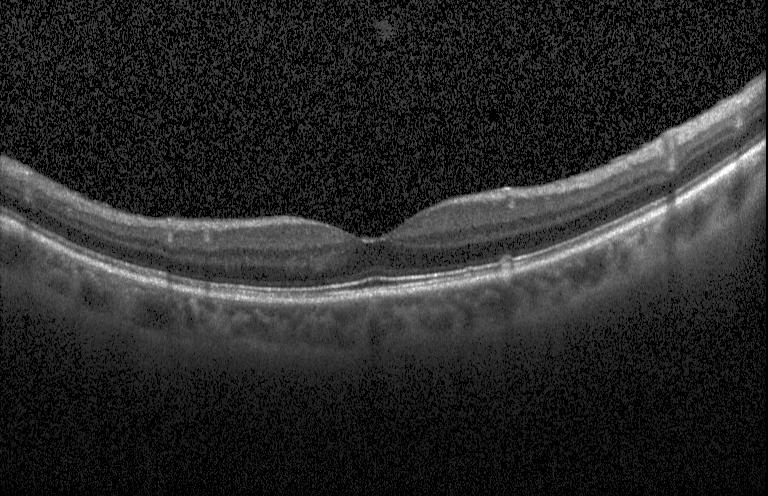 Optical coherence tomography B-scan. Assessment: no evidence of choroidal neovascularization, diabetic macular edema, or drusen.